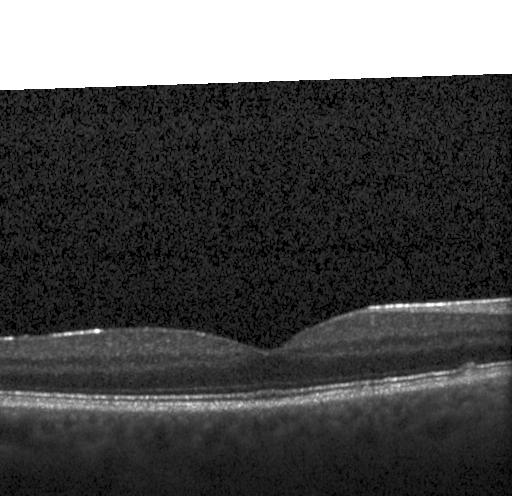 Impression: multiple drusen.